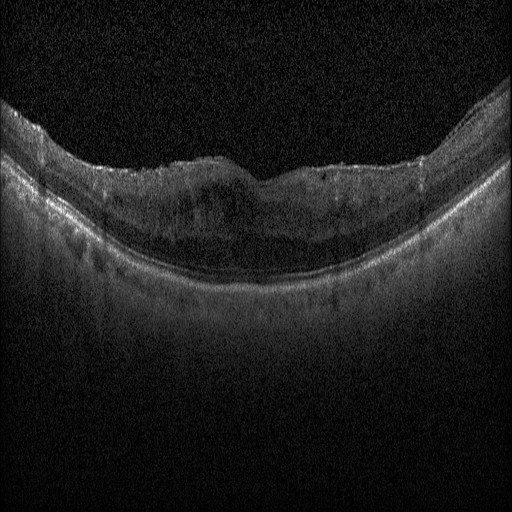

Retinal OCT cross-section. Spectral-domain OCT. Fovea-centered. Instrument: Heidelberg Spectralis.
Dx: DME.